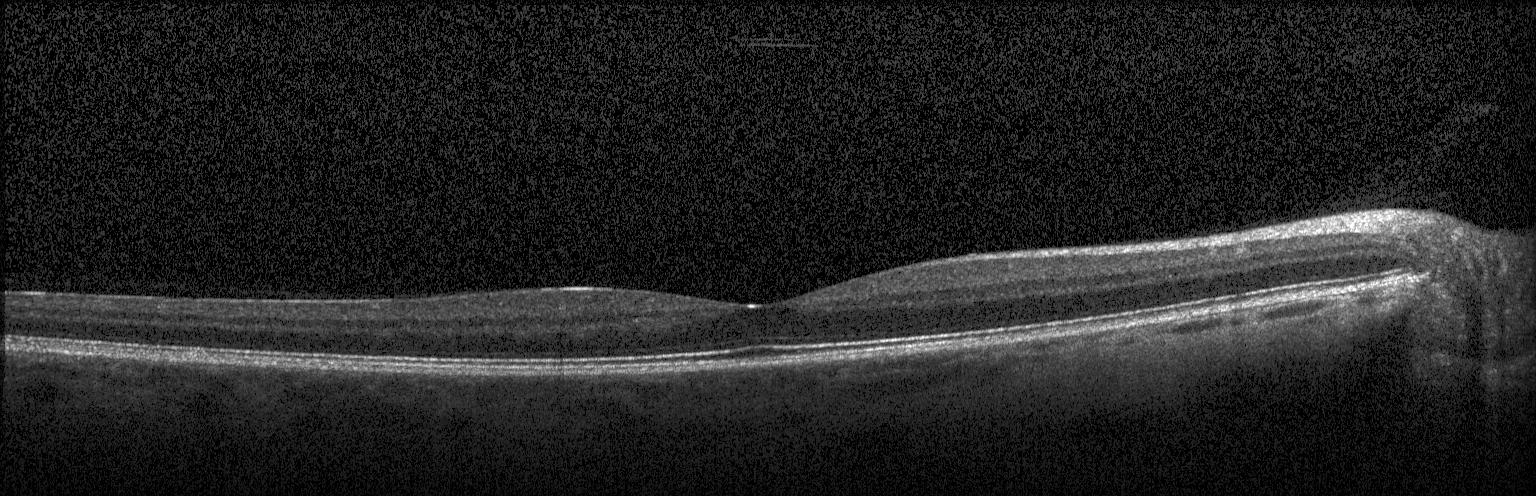 Optical coherence tomography scan
Diagnosis: no choroidal neovascularization, diabetic macular edema, or drusen.